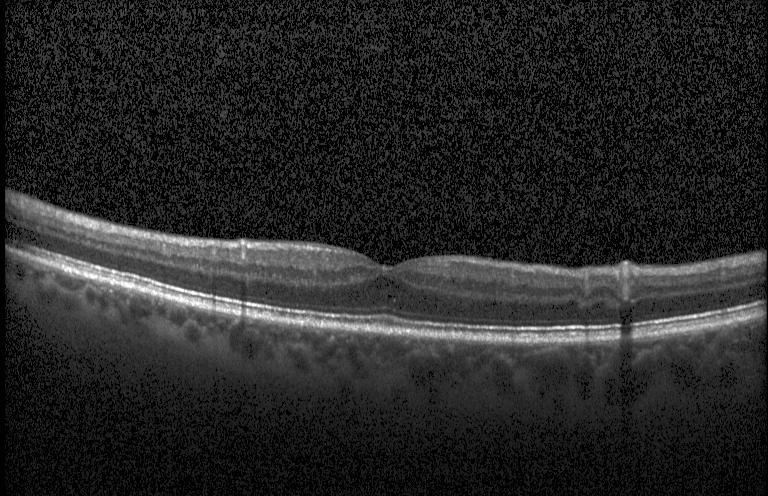 OCT finding: no CNV, DME, or drusen.